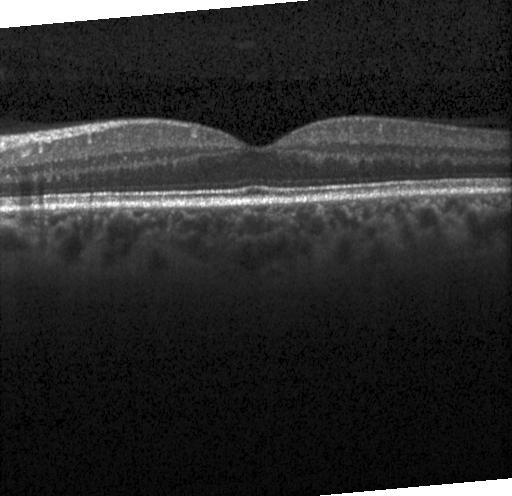 Spectral-domain OCT; retinal OCT B-scan; through the macula. The scan shows neither choroidal neovascularization, diabetic macular edema, nor drusen.